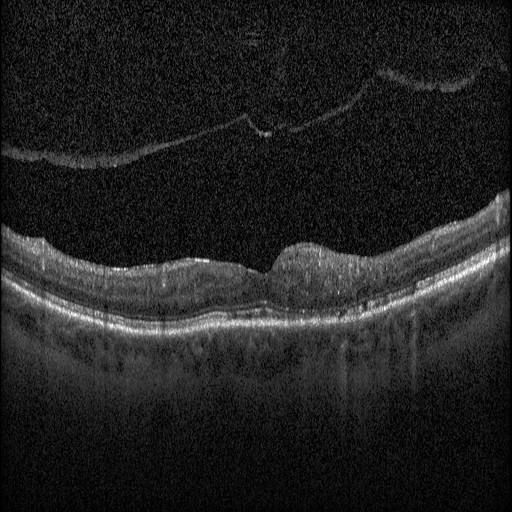
Retinal OCT B-scan — Assessment: diabetic macular edema (DME).